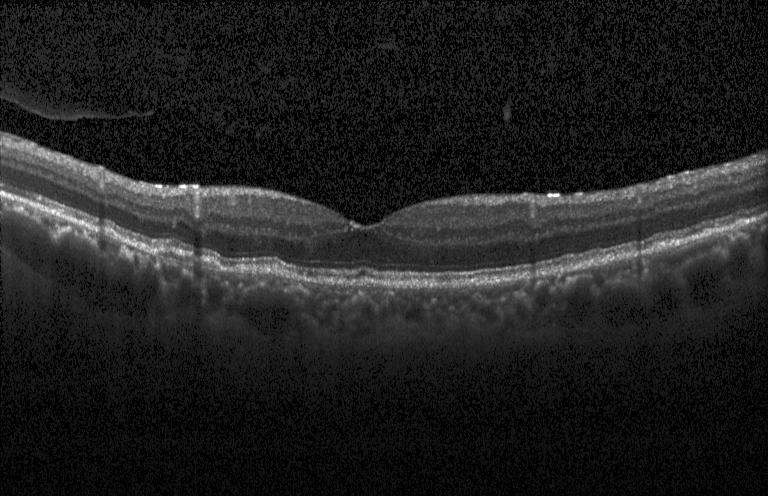

Centered on the fovea · retinal OCT cross-section · Heidelberg Spectralis · spectral-domain OCT. Impression: multiple drusen.